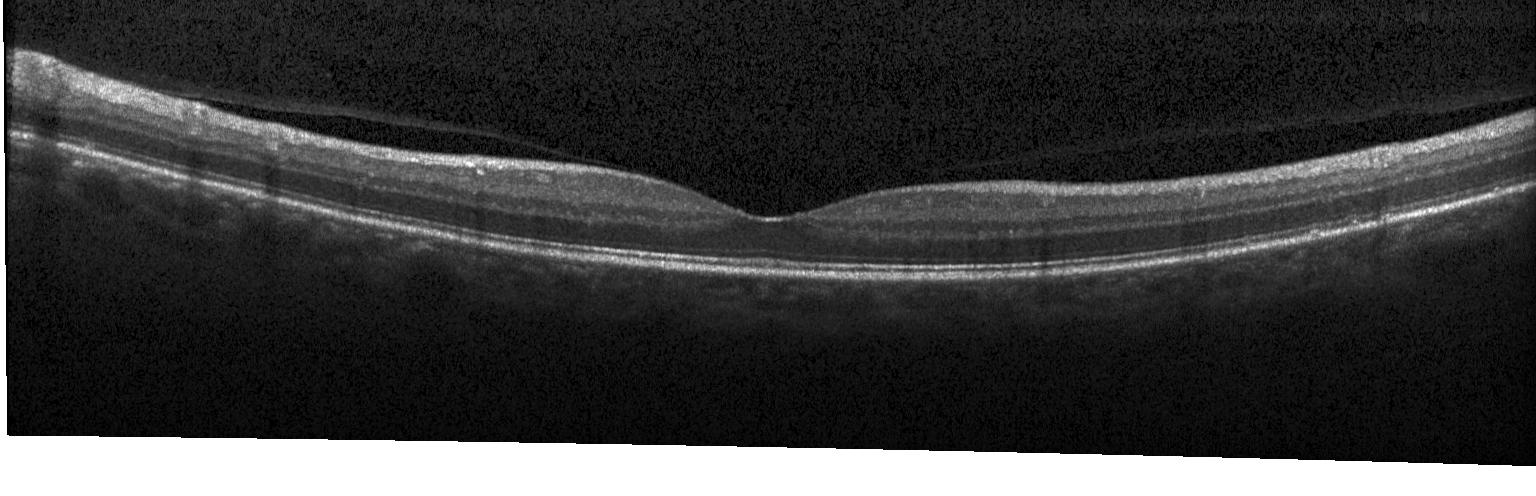
OCT line scan — This B-scan demonstrates no evidence of choroidal neovascularization, diabetic macular edema, or drusen.